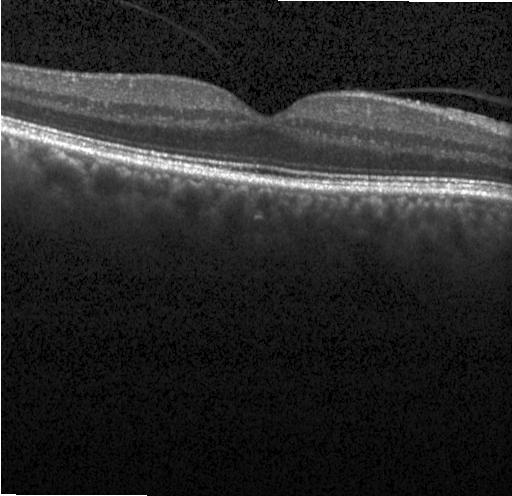

Retinal OCT B-scan · SD-OCT.
Assessment: no evidence of CNV, DME, or drusen.